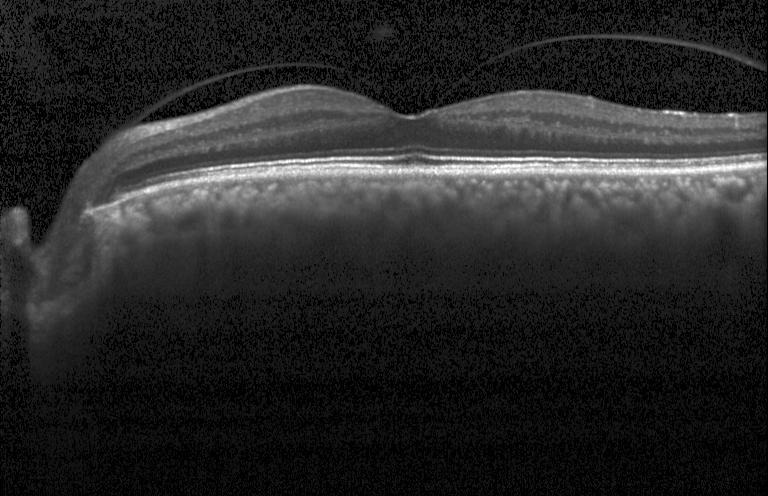 OCT line scan. Diagnosis: no CNV, DME, or drusen.